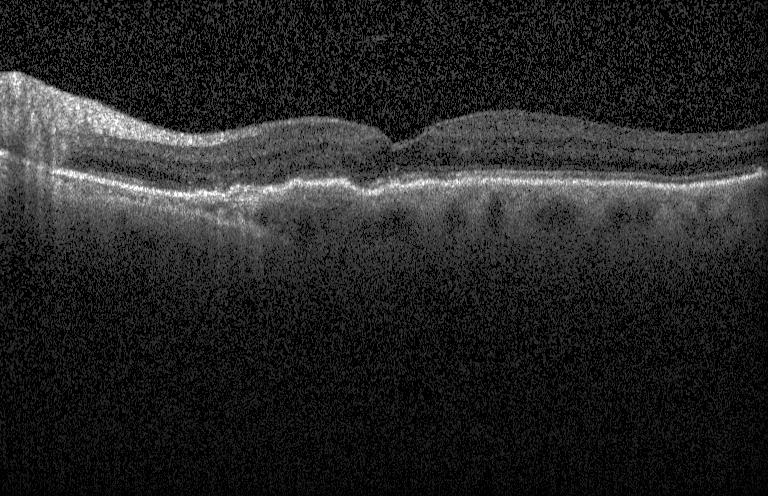
Dx: a choroidal neovascular membrane.